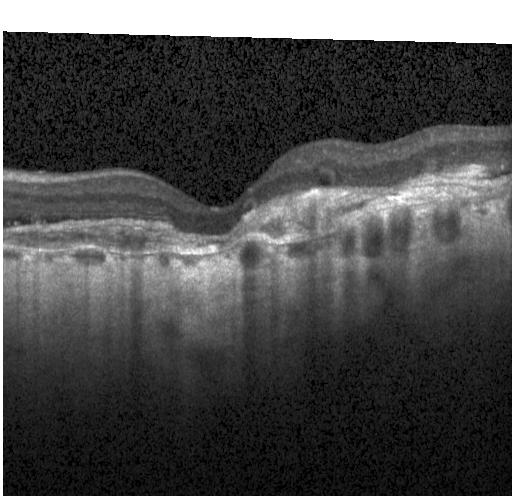

Retinal OCT B-scan, spectral-domain optical coherence tomography
This B-scan demonstrates a choroidal neovascular membrane.